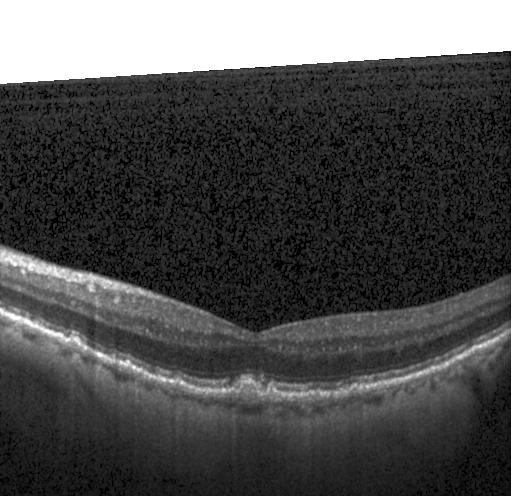
Retinal OCT B-scan.
Impression: drusen.